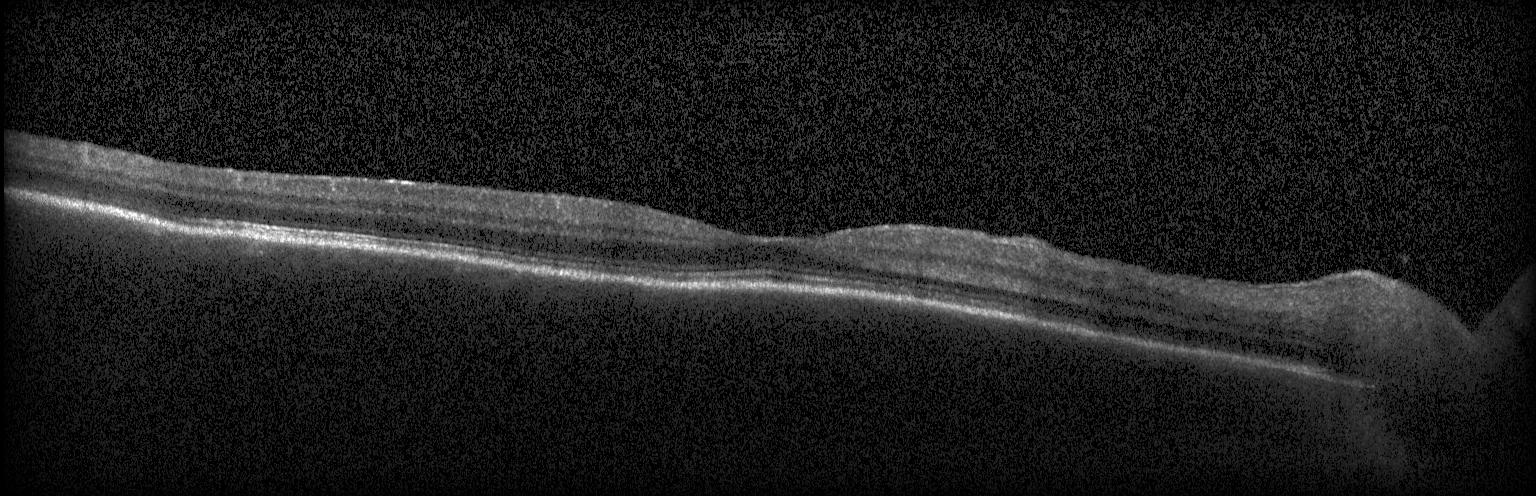

Instrument: Heidelberg Spectralis; OCT line scan; horizontal scan through the fovea — Diagnosis: no evidence of CNV, DME, or drusen.